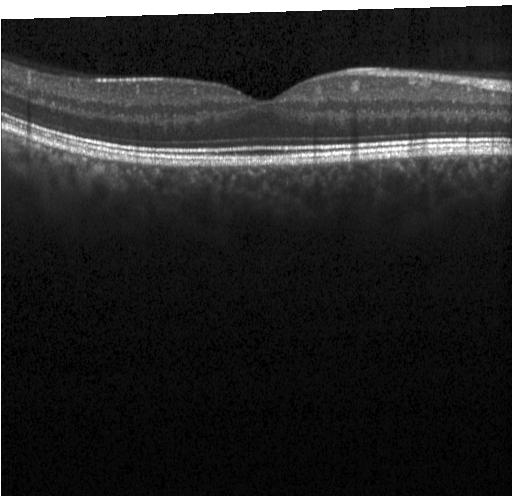 Finding: neither CNV, DME, nor drusen.